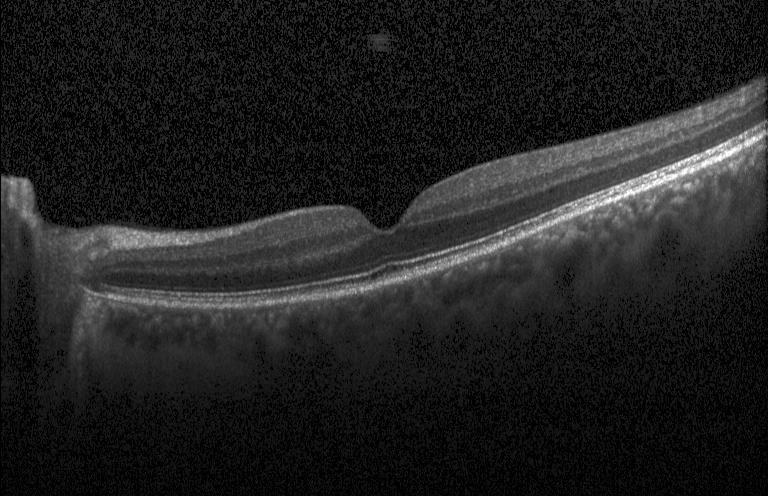 Impression: neither choroidal neovascularization, diabetic macular edema, nor drusen.